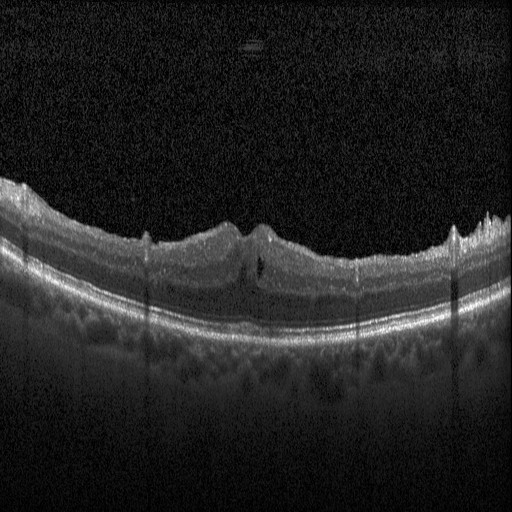 Impression: diabetic macular edema (DME).